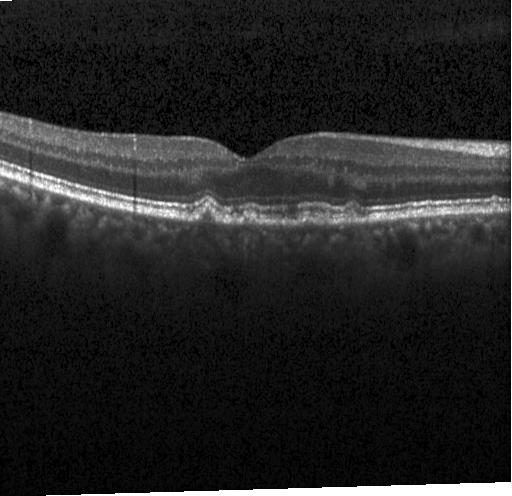 Heidelberg Spectralis OCT system, fovea-centered, SD-OCT, retinal OCT cross-section. Dx: multiple drusen.